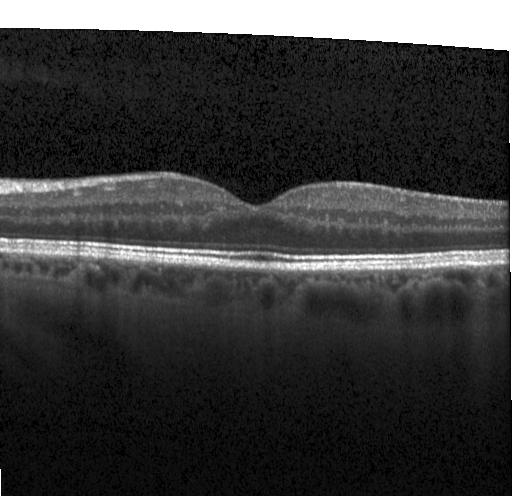

Optical coherence tomography B-scan.
The scan shows neither CNV, DME, nor drusen.